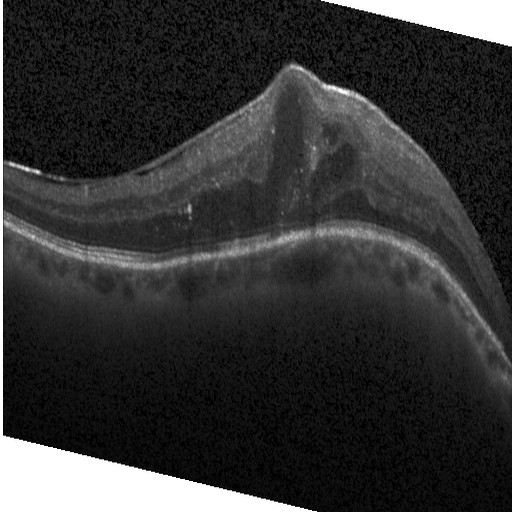 OCT line scan; Heidelberg Spectralis; spectral-domain OCT.
This B-scan demonstrates DME.